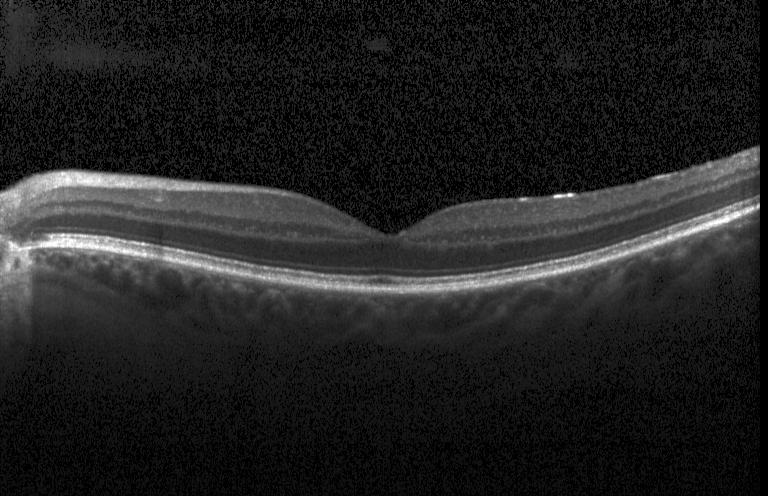

Impression: neither CNV, DME, nor drusen.